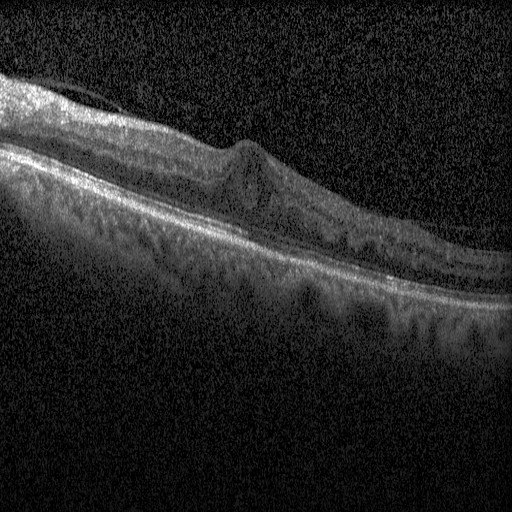
Heidelberg Spectralis, spectral-domain OCT, retinal OCT cross-section, macular scan — The scan shows DME.